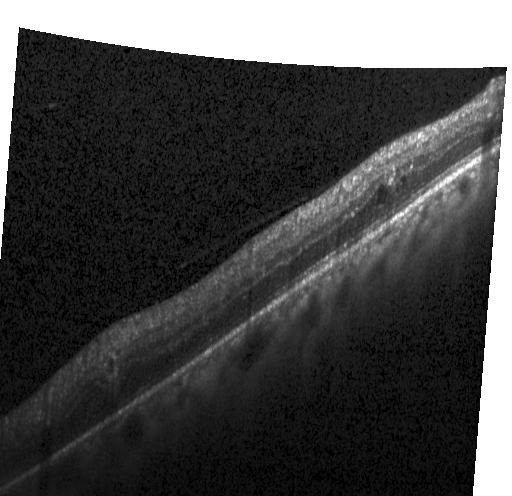 Spectral-domain OCT; OCT line scan.
Diagnosis: DME.